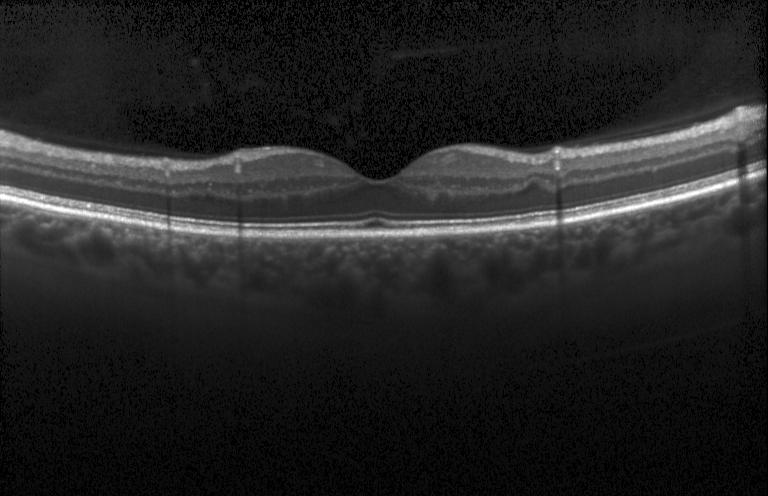
OCT B-scan showing no choroidal neovascularization, diabetic macular edema, or drusen.